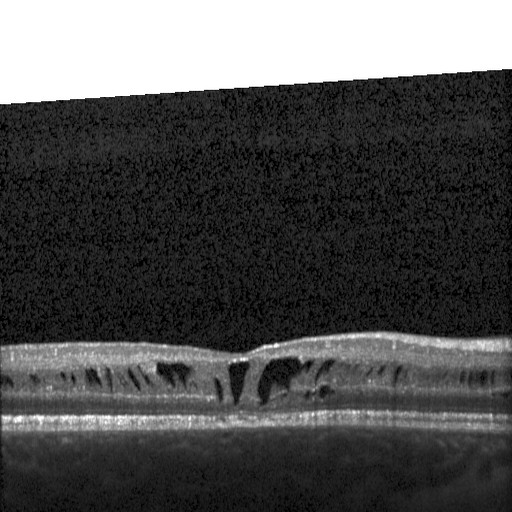
OCT finding: DME.